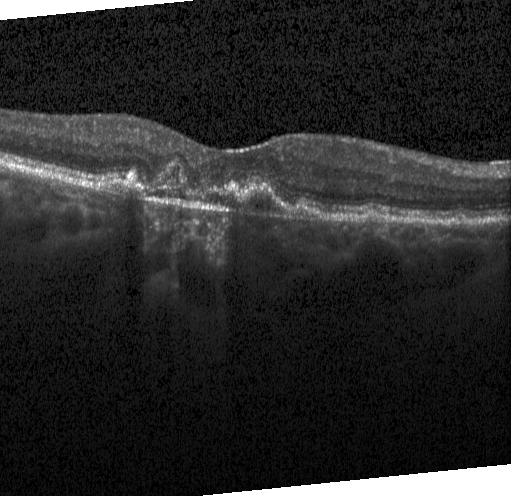 OCT B-scan
Assessment: a choroidal neovascular membrane.